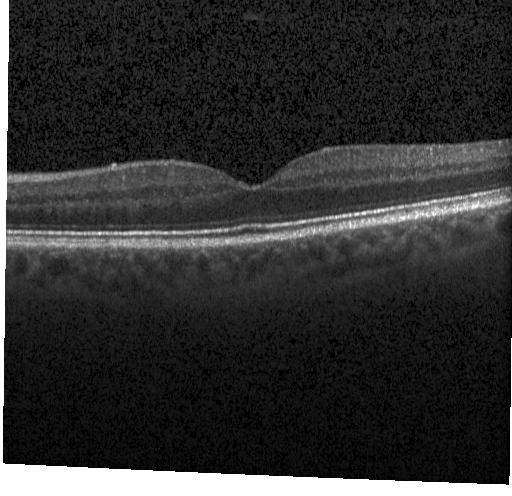 Heidelberg Spectralis OCT system, OCT B-scan, SD-OCT, centered on the fovea. Finding: neither choroidal neovascularization, diabetic macular edema, nor drusen.